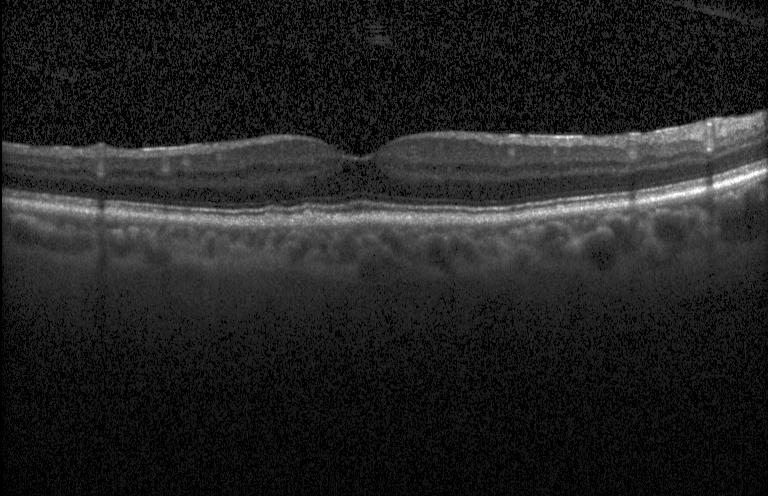 Retinal OCT cross-section showing sub-RPE drusenoid deposits.